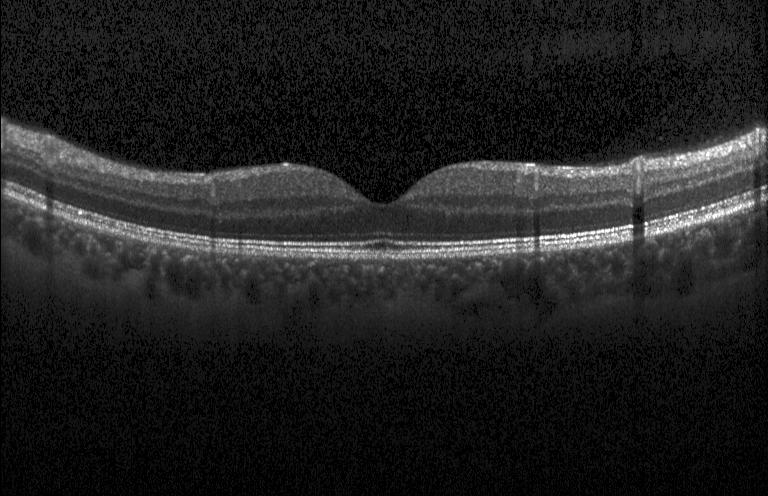
SD-OCT · retinal OCT cross-section · acquired on a Heidelberg Spectralis · centered on the fovea.
Finding: no choroidal neovascularization, no diabetic macular edema, and no drusen.